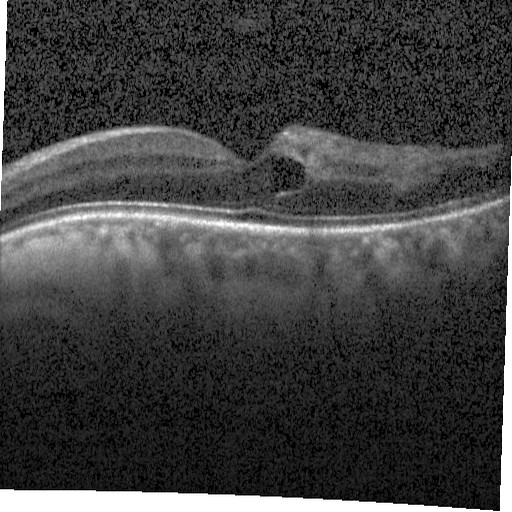 Through the macula. Spectral-domain OCT. Retinal OCT cross-section — Diagnosis: DME.